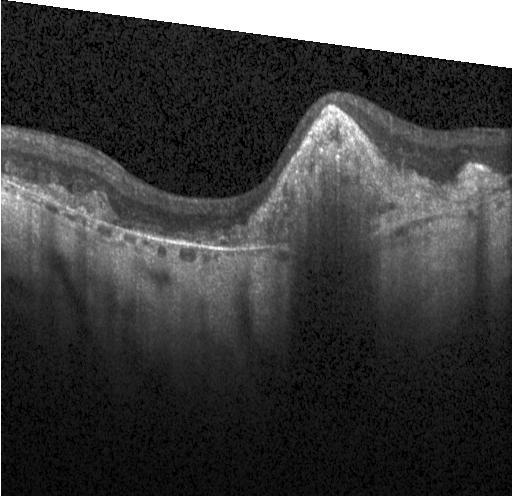 Optical coherence tomography B-scan.
Impression: a choroidal neovascular membrane.